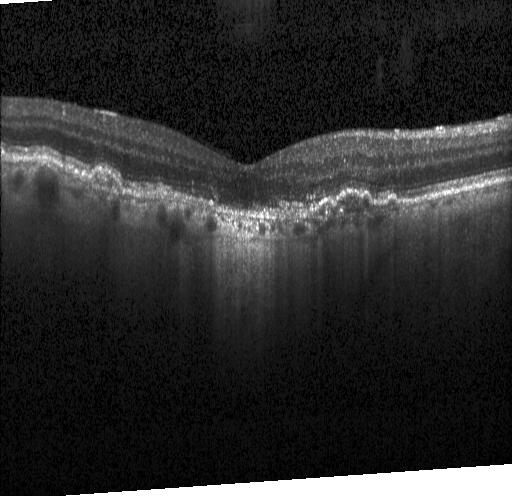 Horizontal scan through the fovea, optical coherence tomography B-scan.
Diagnosis: a choroidal neovascular membrane.